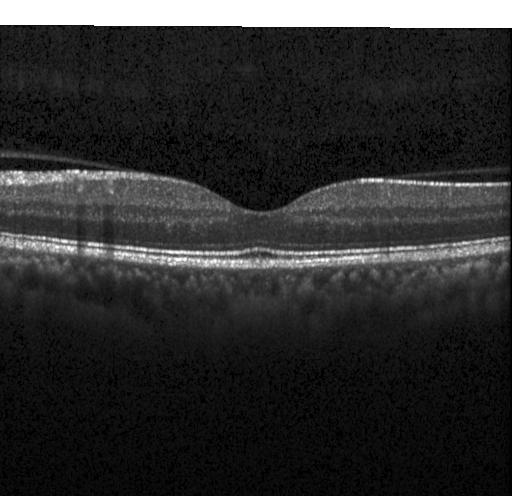
SD-OCT; optical coherence tomography B-scan; horizontal scan through the fovea; instrument: Heidelberg Spectralis — Diagnosis: no choroidal neovascularization, diabetic macular edema, or drusen.